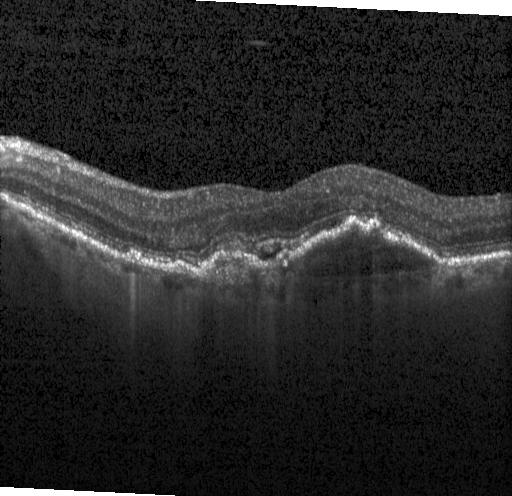
Spectral-domain OCT; optical coherence tomography scan; acquired on a Heidelberg Spectralis; through the macula. CNV.